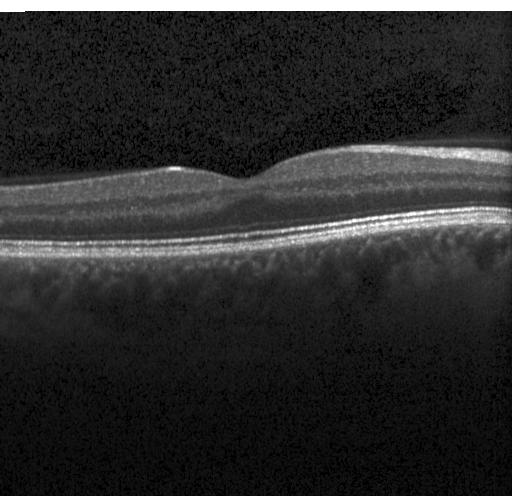 This B-scan demonstrates no CNV, no DME, and no drusen.